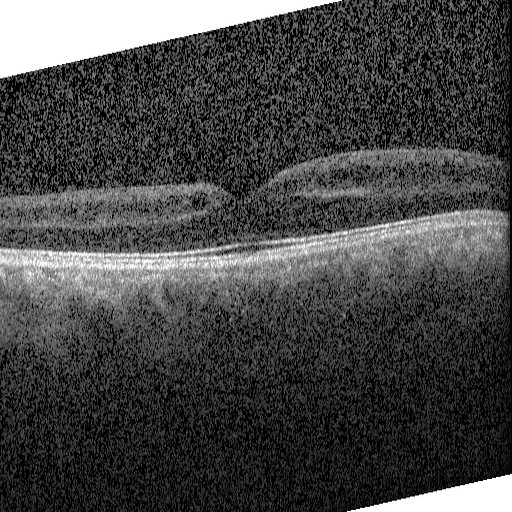 Optical coherence tomography scan · spectral-domain OCT · acquired on a Heidelberg Spectralis.
Diabetic macular edema (DME).